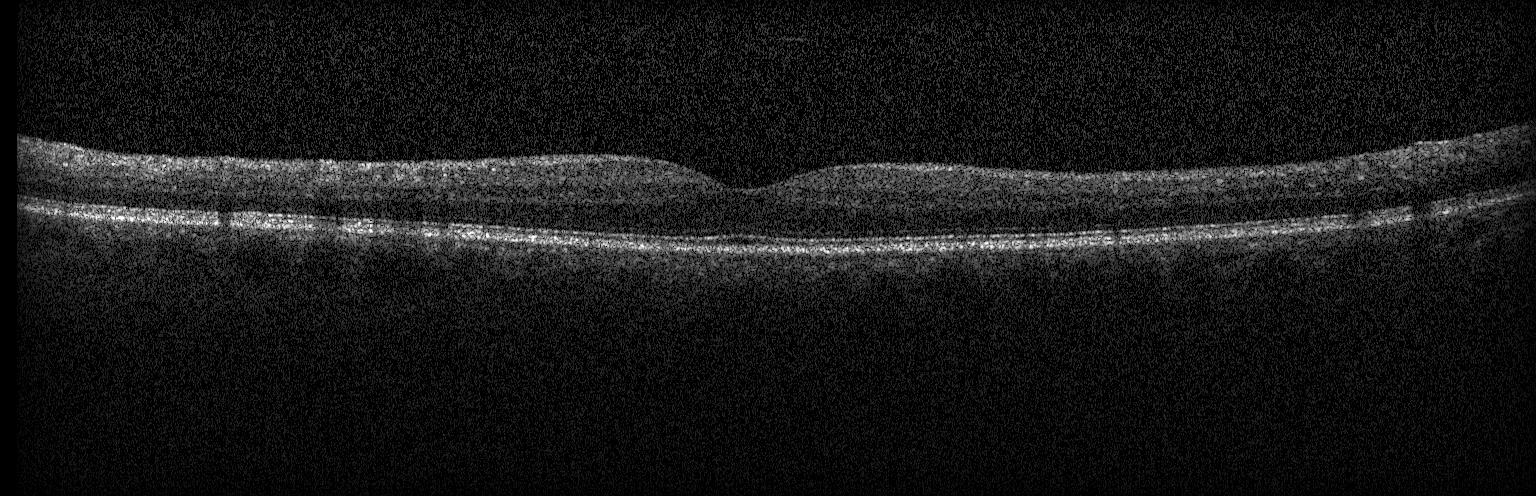 Spectral-domain OCT B-scan: no CNV, no DME, and no drusen.